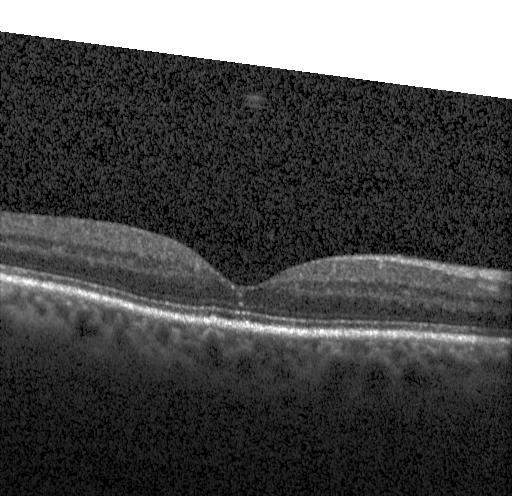
Diagnosis: neither choroidal neovascularization, diabetic macular edema, nor drusen.